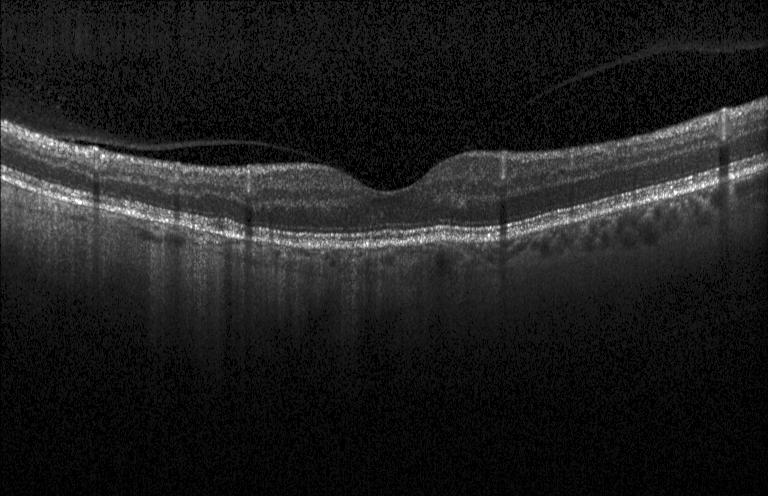
Retinal OCT B-scan. Diagnosis: no CNV, DME, or drusen.